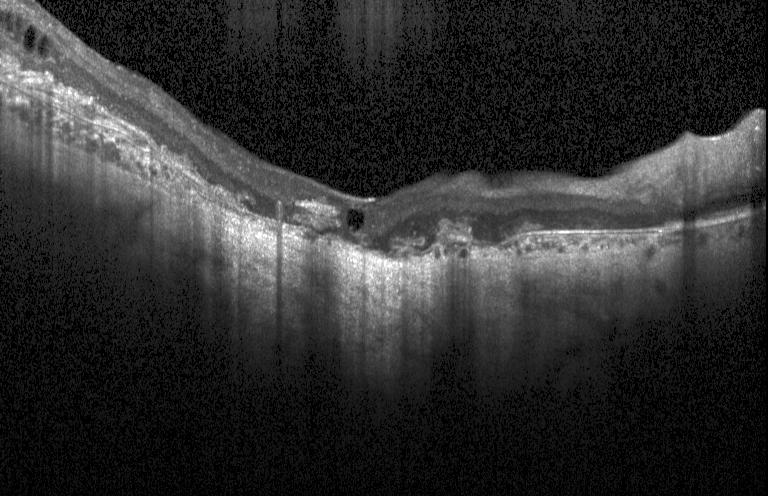

Macular OCT: a choroidal neovascular membrane.